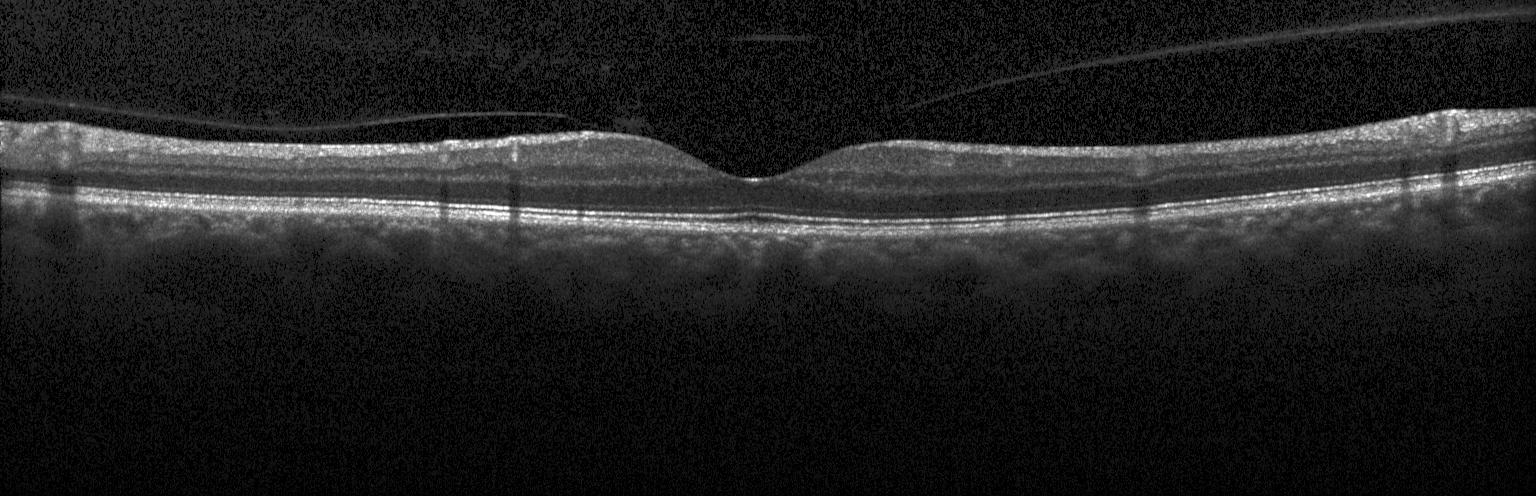

OCT finding: no evidence of CNV, DME, or drusen.